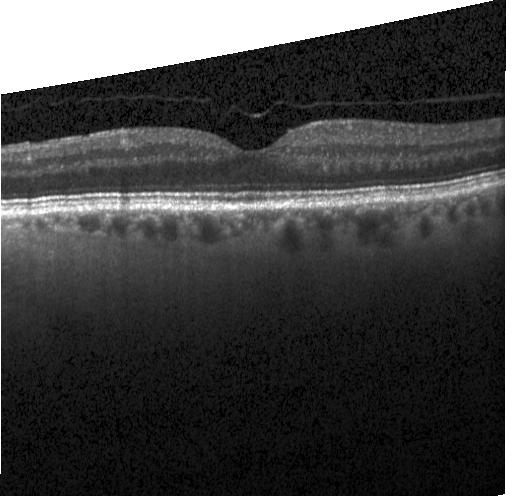 Optical coherence tomography B-scan.
Dx: no CNV, no DME, and no drusen.